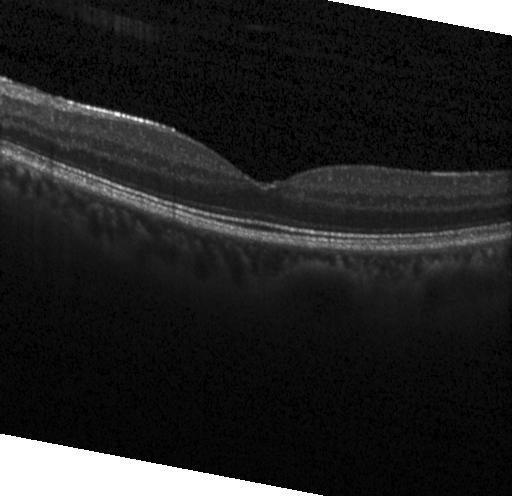
Spectral-domain OCT. OCT line scan.
The scan shows no evidence of CNV, DME, or drusen.